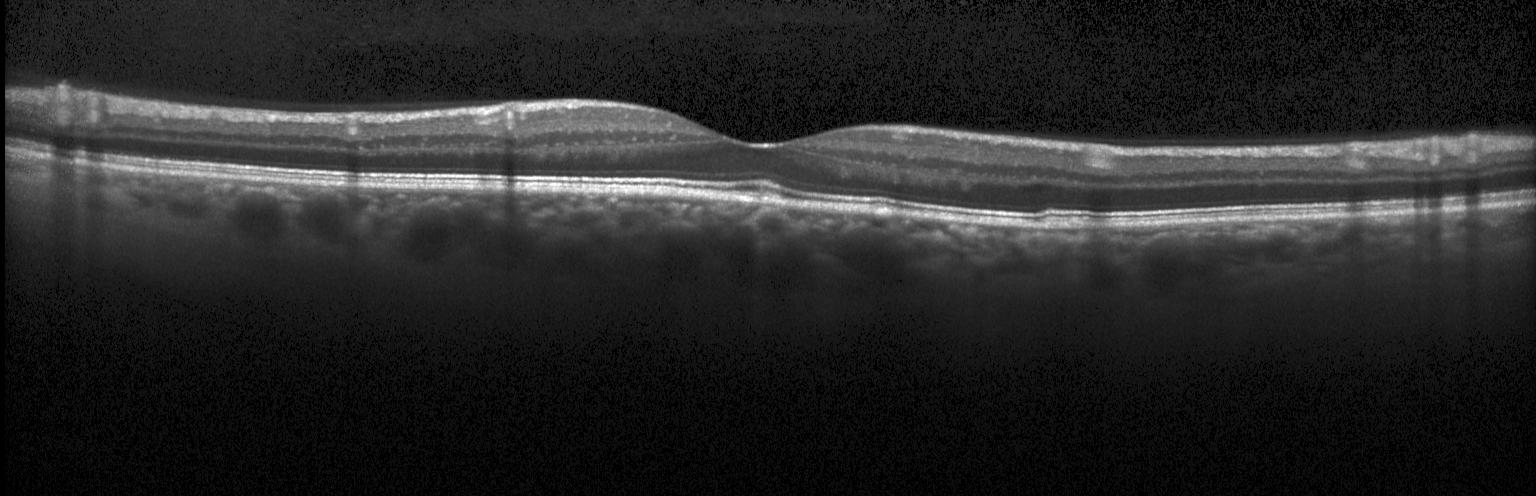
Retinal OCT cross-section showing no CNV, DME, or drusen.